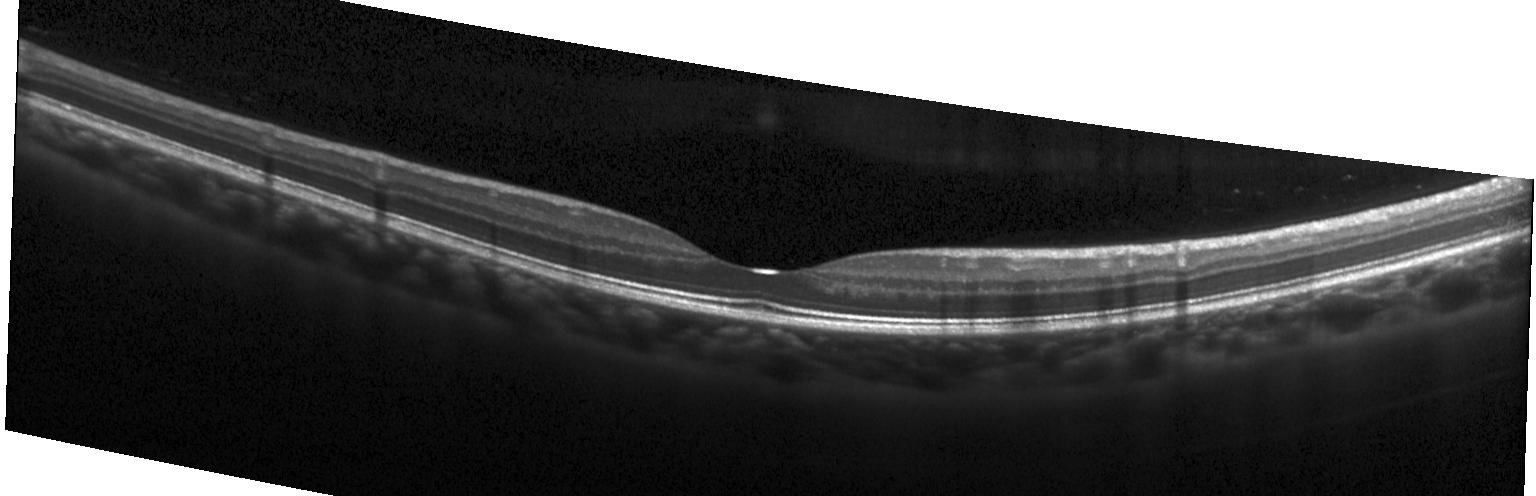
OCT B-scan showing neither CNV, DME, nor drusen.